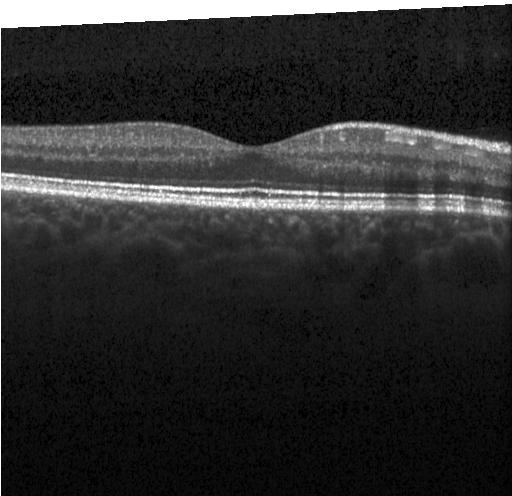
OCT B-scan. Through the macula. Heidelberg Spectralis OCT system.
Assessment: no CNV, no DME, and no drusen.